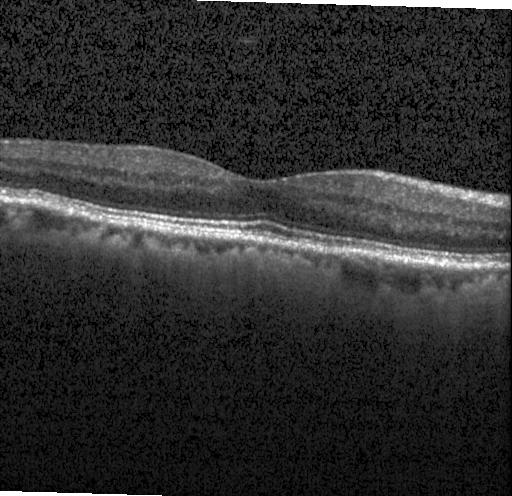

Optical coherence tomography scan · horizontal scan through the fovea · spectral-domain optical coherence tomography · instrument: Heidelberg Spectralis
Finding: no choroidal neovascularization, no diabetic macular edema, and no drusen.